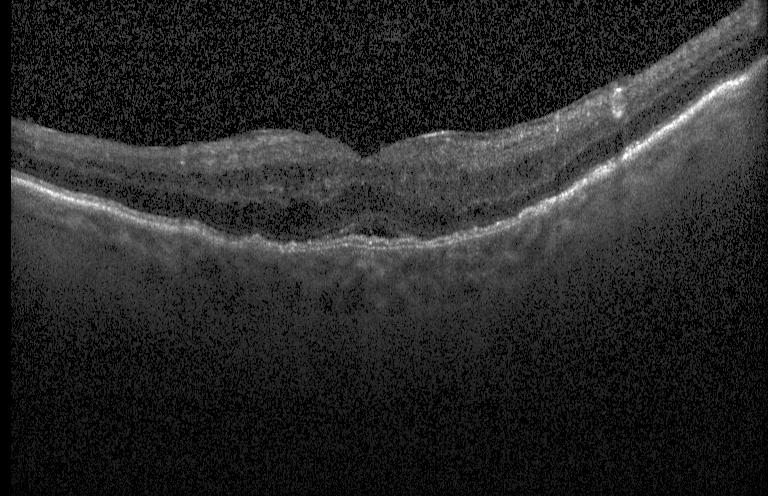
Assessment: CNV.